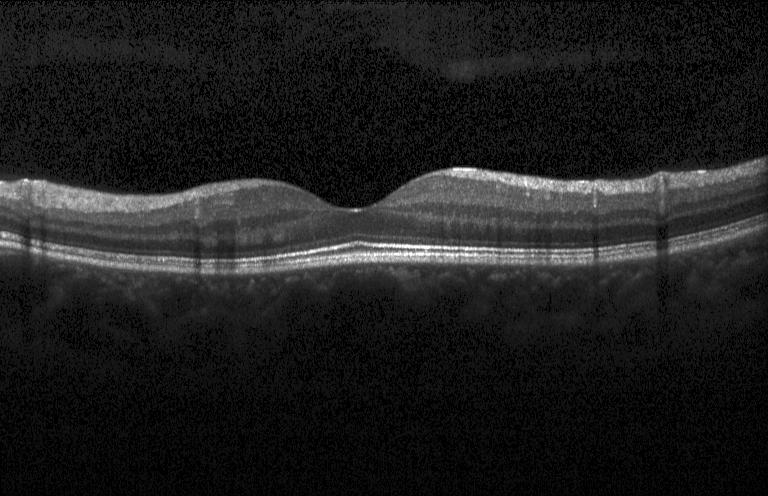 Finding: no choroidal neovascularization, no diabetic macular edema, and no drusen.